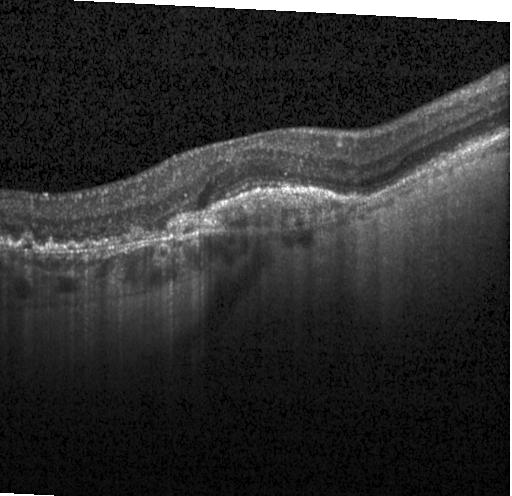
SD-OCT · OCT line scan · instrument: Heidelberg Spectralis · centered on the fovea. A choroidal neovascular membrane.